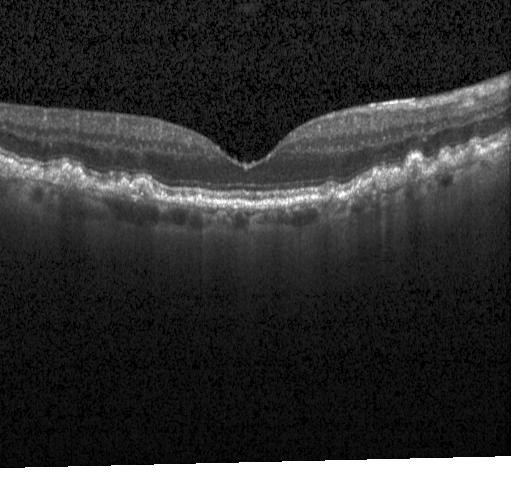 Macular OCT demonstrating sub-RPE drusenoid deposits.